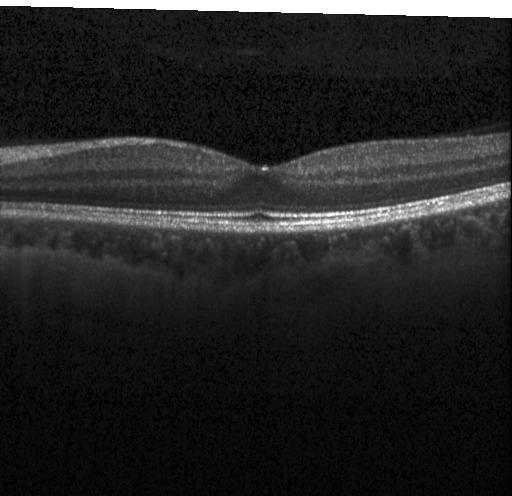

OCT line scan. Macular scan. Instrument: Heidelberg Spectralis. Spectral-domain OCT — Dx: neither choroidal neovascularization, diabetic macular edema, nor drusen.